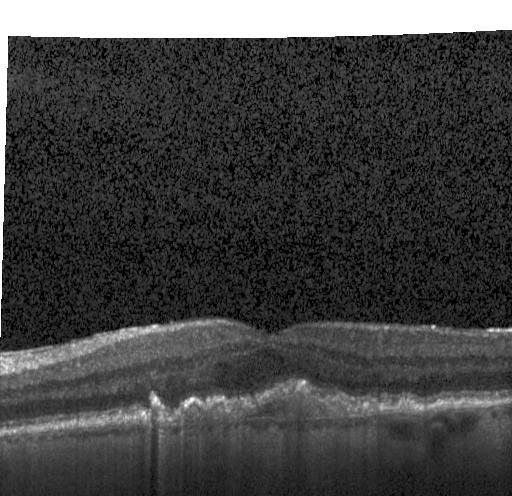 Spectral-domain OCT · through the macula · OCT B-scan.
Diagnosis: a choroidal neovascular membrane.